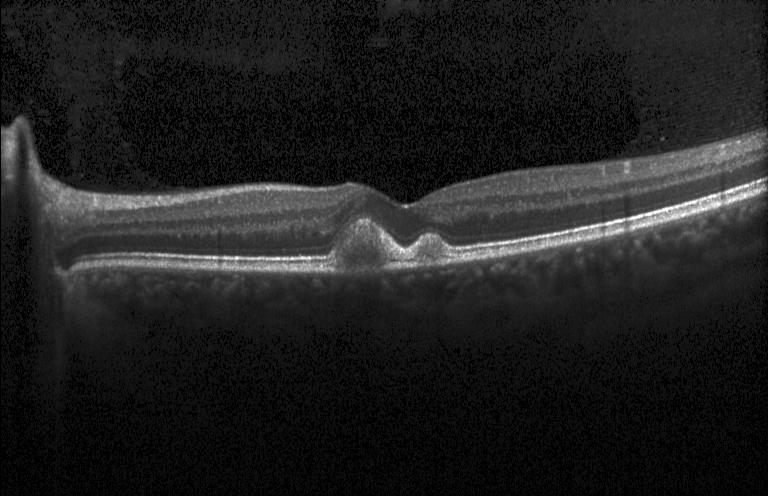
OCT finding: drusen.